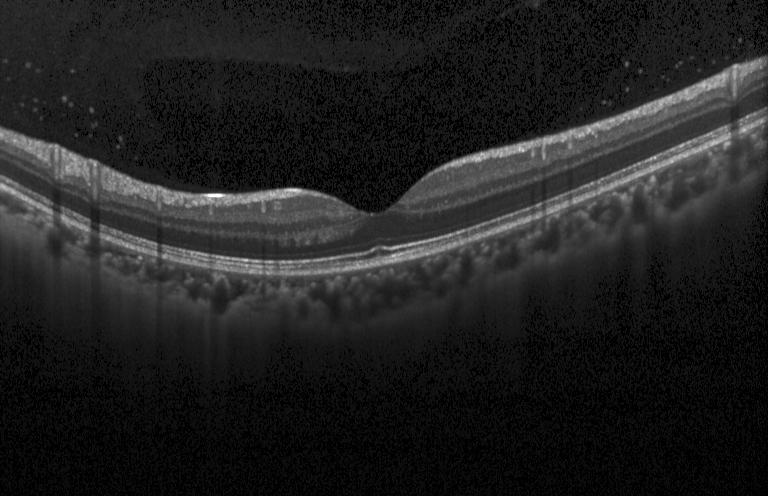

SD-OCT. Retinal OCT B-scan.
The scan shows no evidence of choroidal neovascularization, diabetic macular edema, or drusen.